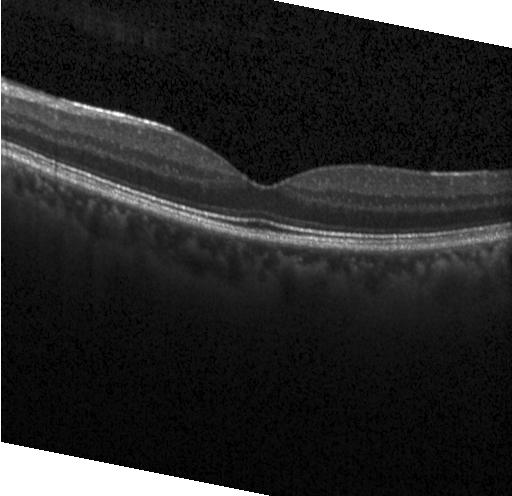 Impression: no choroidal neovascularization, diabetic macular edema, or drusen.